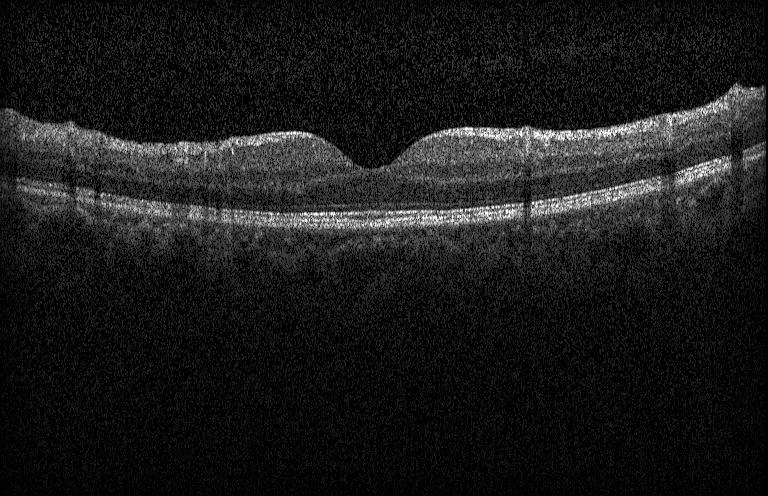 Optical coherence tomography scan; instrument: Heidelberg Spectralis; spectral-domain optical coherence tomography; horizontal scan through the fovea — Finding: no choroidal neovascularization, diabetic macular edema, or drusen.